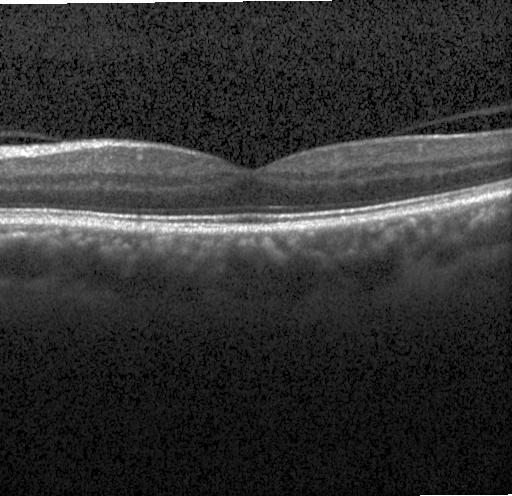

OCT line scan. SD-OCT
Assessment: no CNV, no DME, and no drusen.